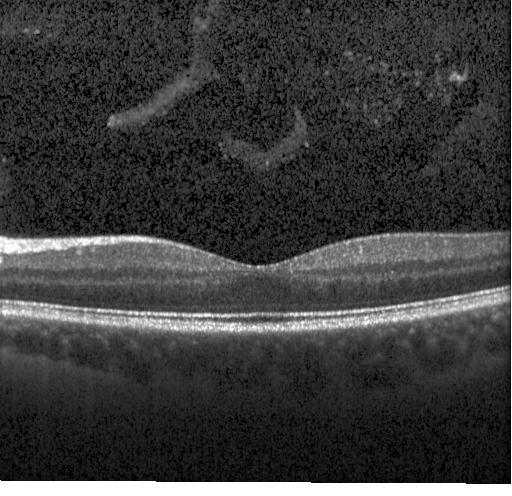
Optical coherence tomography B-scan.
Diagnosis: neither CNV, DME, nor drusen.